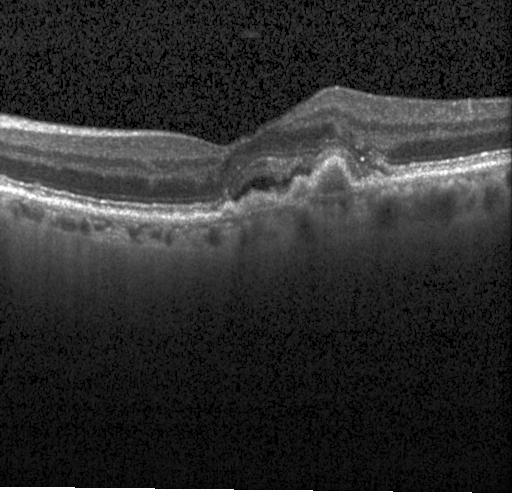 Finding: choroidal neovascularization.